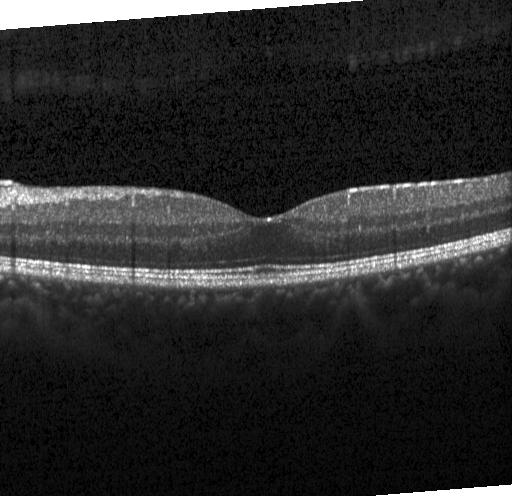
Impression: no choroidal neovascularization, diabetic macular edema, or drusen.